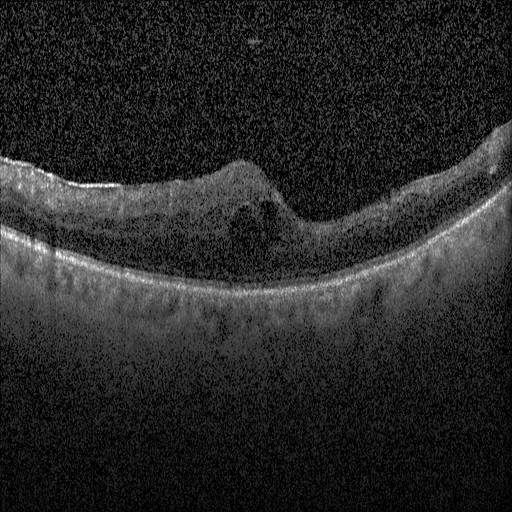
Diabetic macular edema.